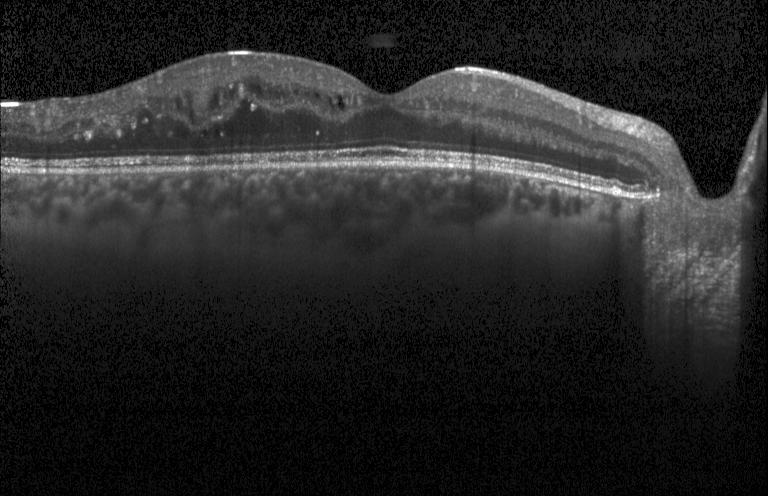
Heidelberg Spectralis OCT system · OCT line scan. OCT finding: diabetic macular edema (DME).